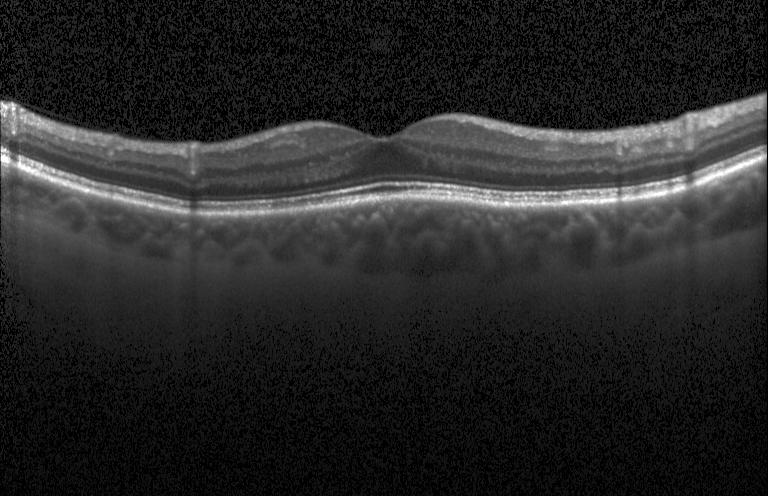

Finding: no evidence of CNV, DME, or drusen.